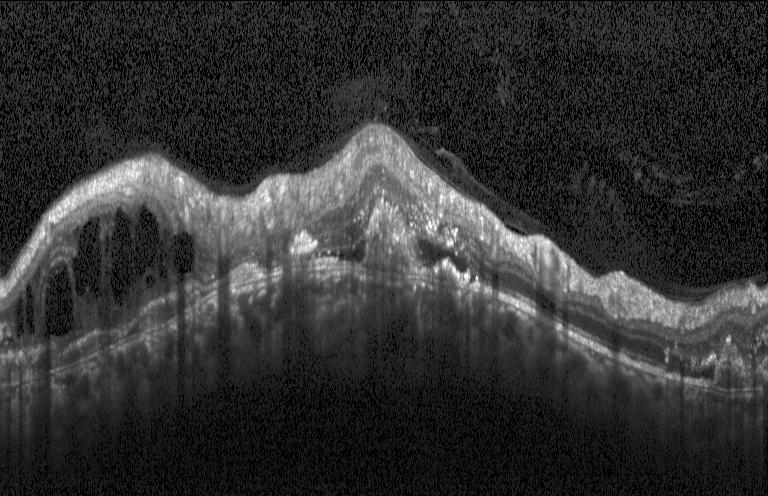 OCT line scan
Impression: CNV.